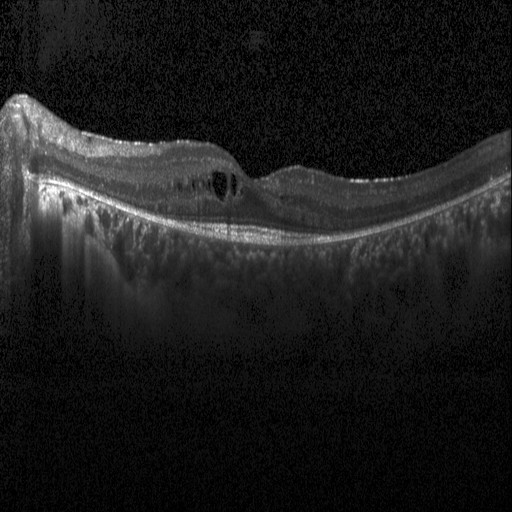

Heidelberg Spectralis; retinal OCT cross-section. The scan shows diabetic macular edema (DME).